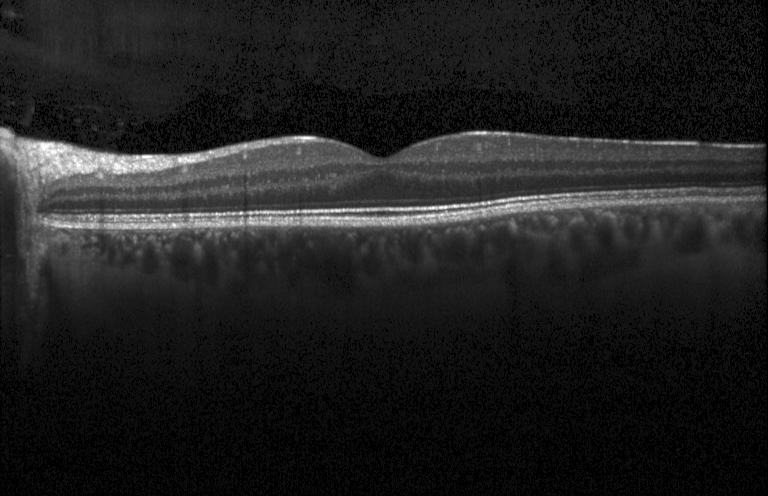 Instrument: Heidelberg Spectralis · macular scan · retinal OCT B-scan. Finding: neither choroidal neovascularization, diabetic macular edema, nor drusen.